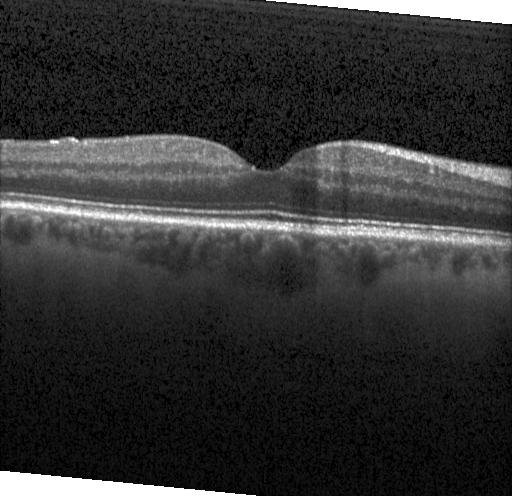
Through the macula · SD-OCT · optical coherence tomography scan. Finding: no evidence of choroidal neovascularization, diabetic macular edema, or drusen.